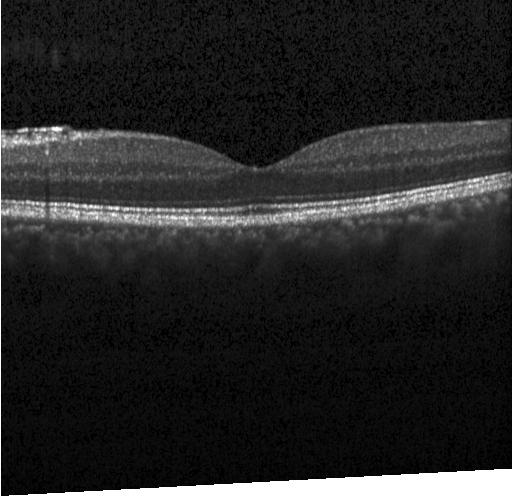 Retinal OCT cross-section
OCT finding: neither CNV, DME, nor drusen.